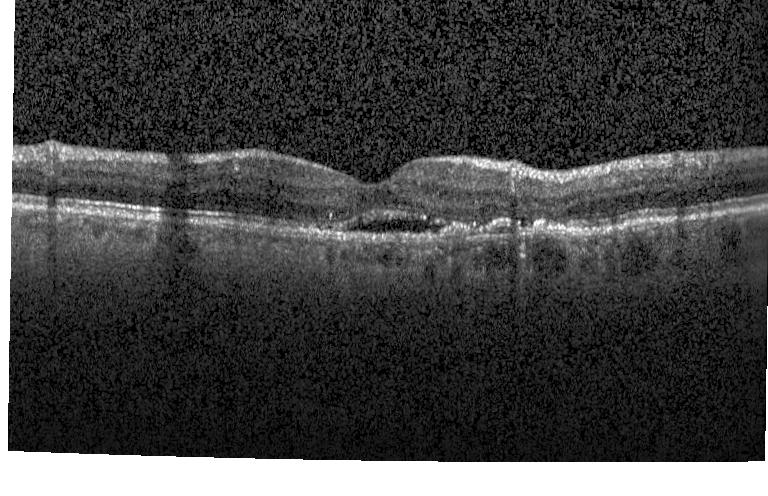
Macular scan, Heidelberg Spectralis OCT system, retinal OCT cross-section
OCT finding: choroidal neovascularization (CNV).